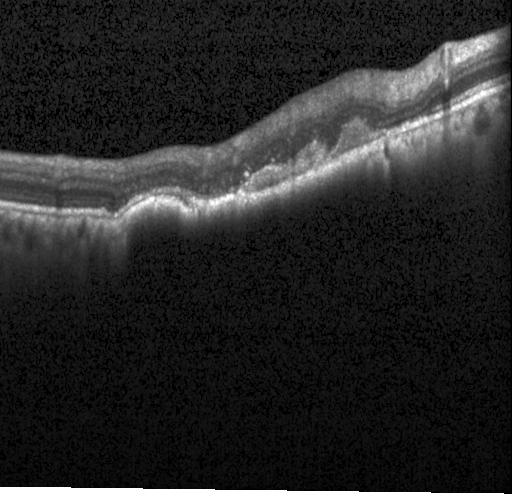 Diagnosis: a choroidal neovascular membrane.